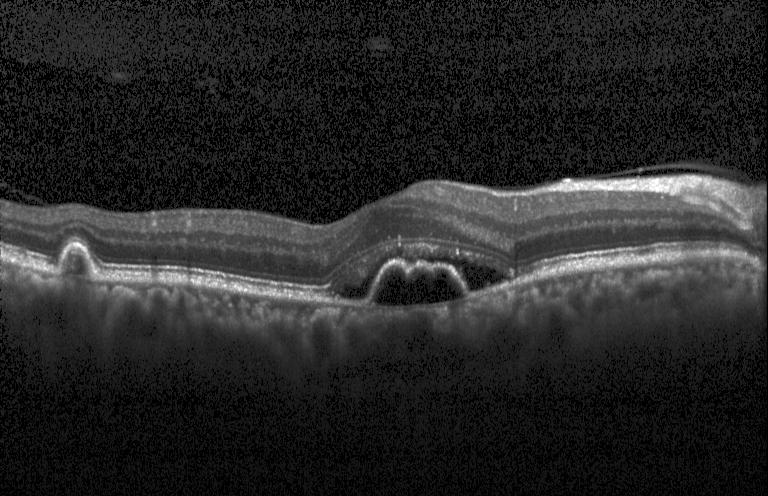

Assessment: choroidal neovascularization.